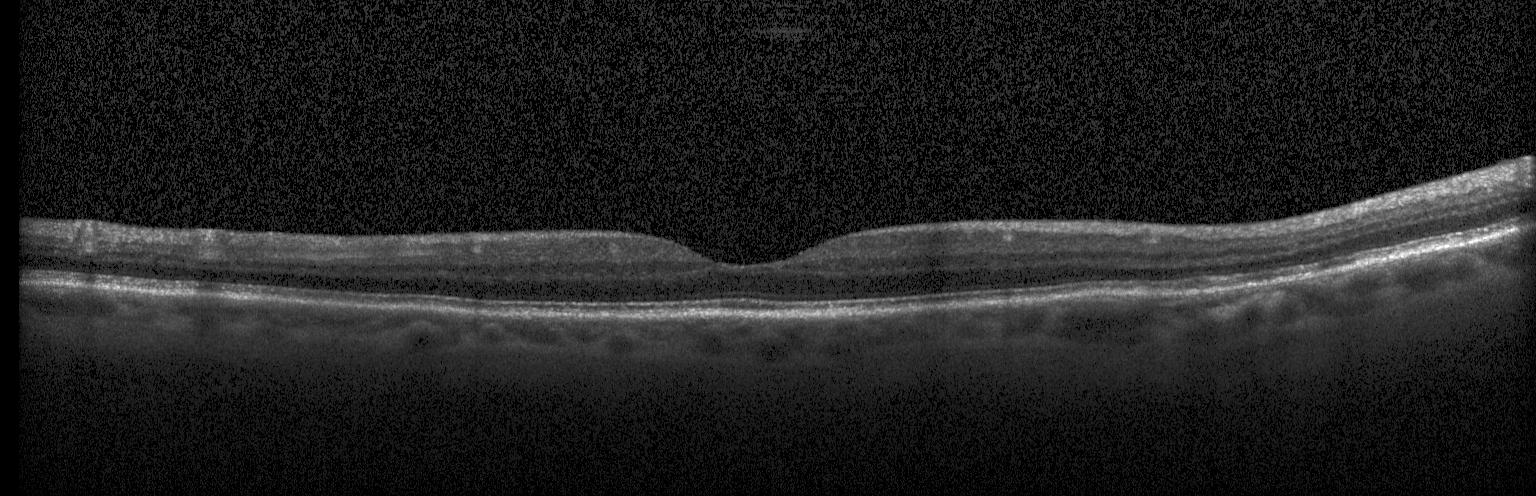
Heidelberg Spectralis OCT system; SD-OCT; fovea-centered; OCT B-scan
No evidence of CNV, DME, or drusen.